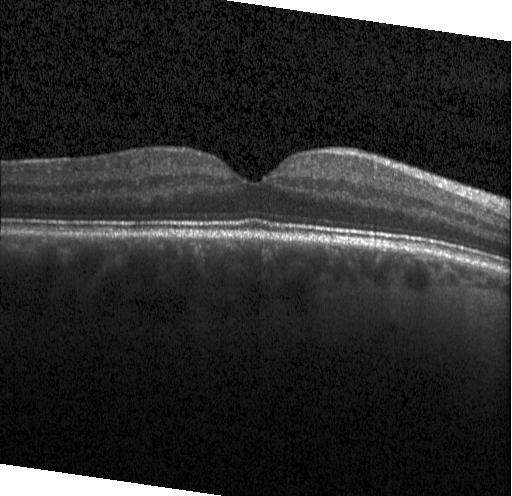

OCT B-scan
Finding: no evidence of choroidal neovascularization, diabetic macular edema, or drusen.